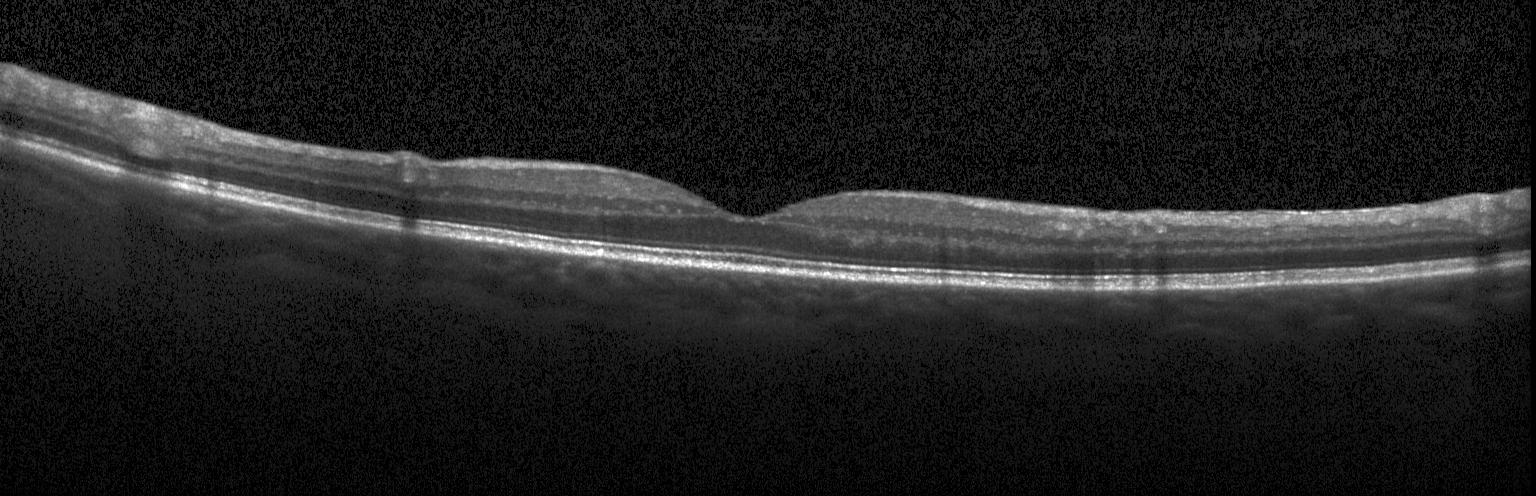
Retinal OCT cross-section. Heidelberg Spectralis OCT system.
This B-scan demonstrates neither choroidal neovascularization, diabetic macular edema, nor drusen.